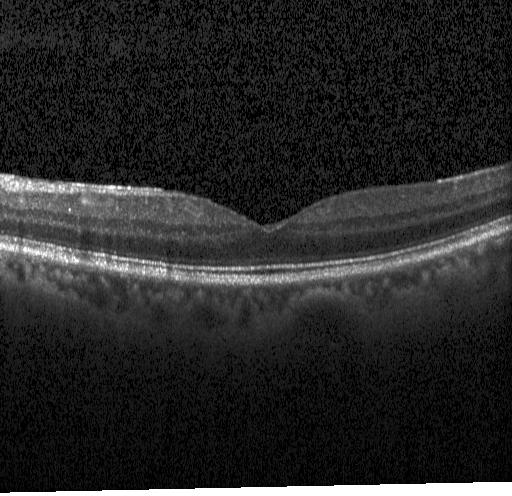 Diagnosis: neither choroidal neovascularization, diabetic macular edema, nor drusen.